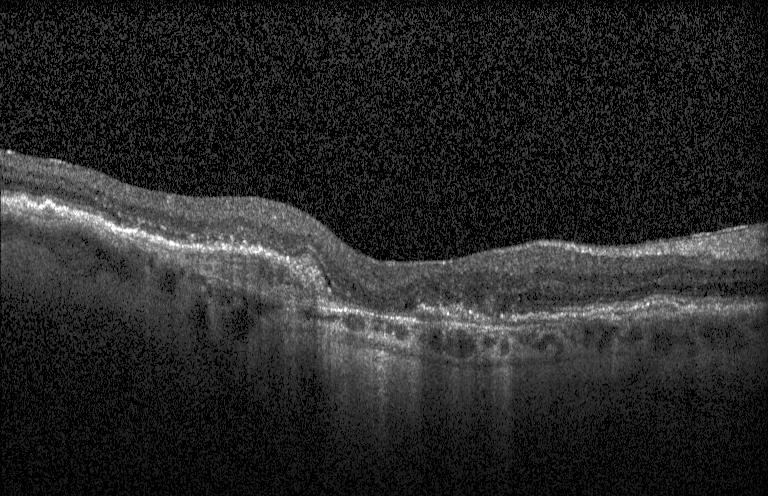
Retinal OCT cross-section · through the macula
A choroidal neovascular membrane.